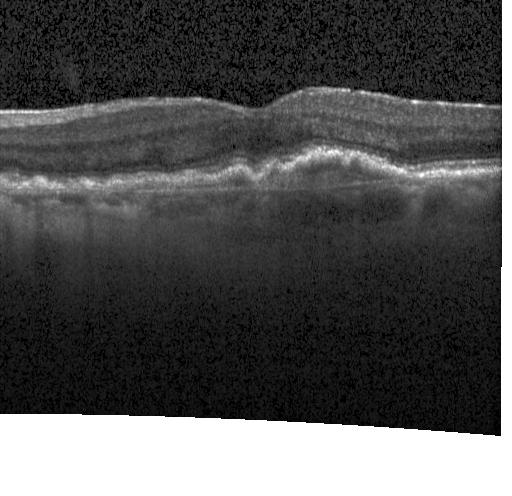 Instrument: Heidelberg Spectralis, spectral-domain optical coherence tomography, OCT B-scan, fovea-centered.
Finding: a choroidal neovascular membrane.